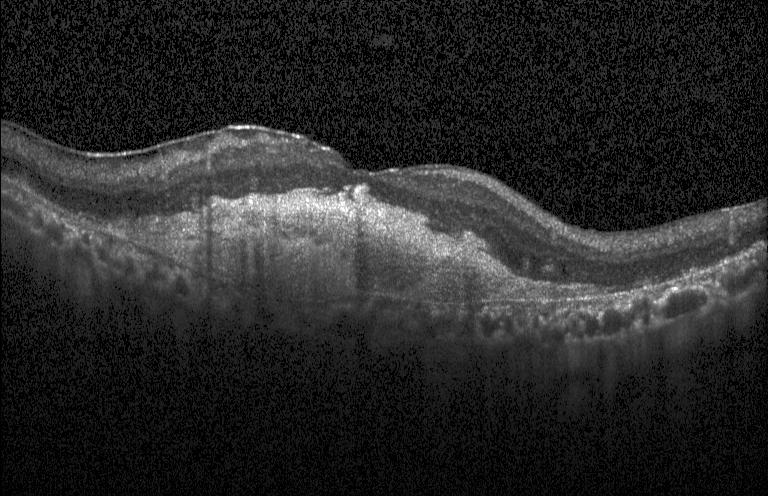

Dx: CNV.